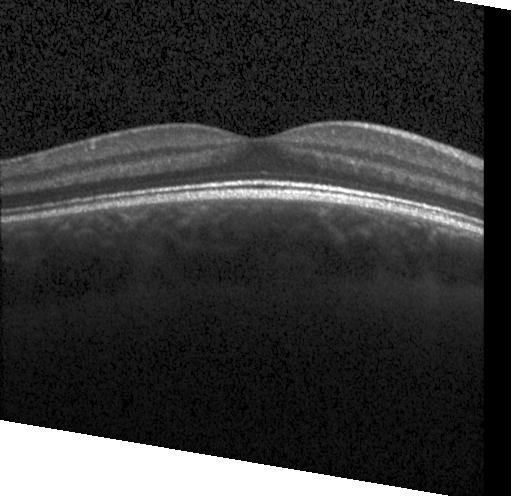 Retinal OCT B-scan; SD-OCT.
Neither choroidal neovascularization, diabetic macular edema, nor drusen.